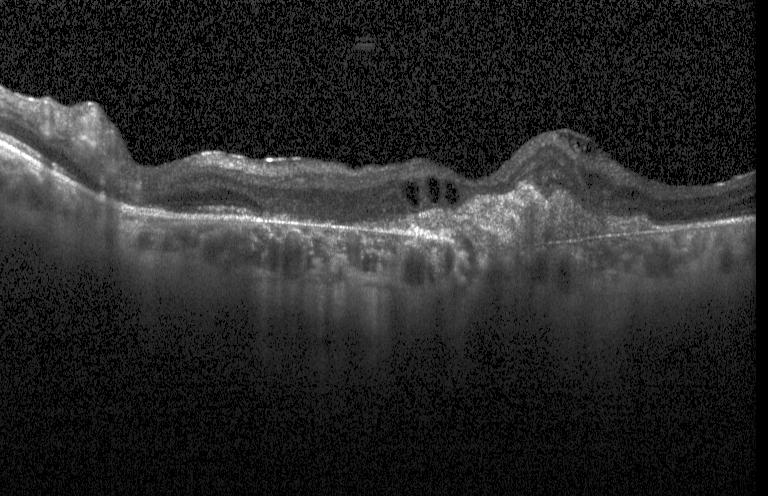
Spectral-domain optical coherence tomography, instrument: Heidelberg Spectralis, centered on the fovea, optical coherence tomography B-scan.
This B-scan demonstrates choroidal neovascularization (CNV).